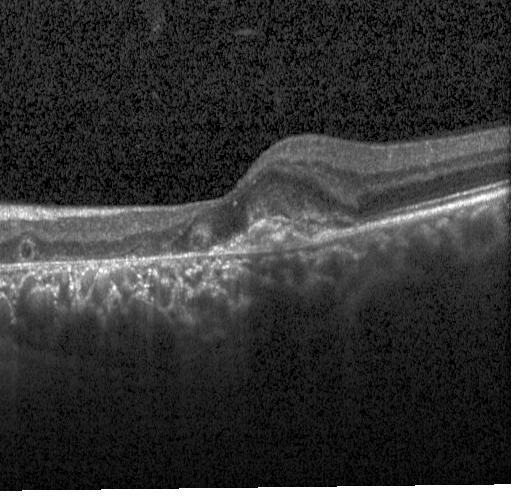
Instrument: Heidelberg Spectralis. Retinal OCT cross-section — Diagnosis: CNV.